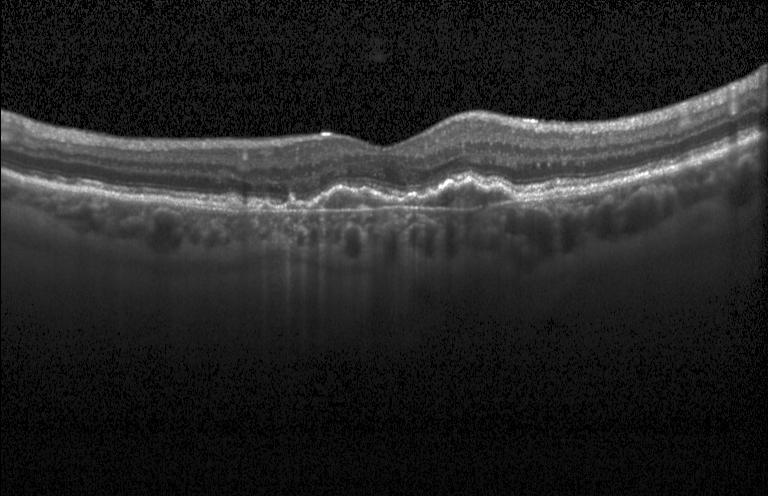 Assessment: a choroidal neovascular membrane.